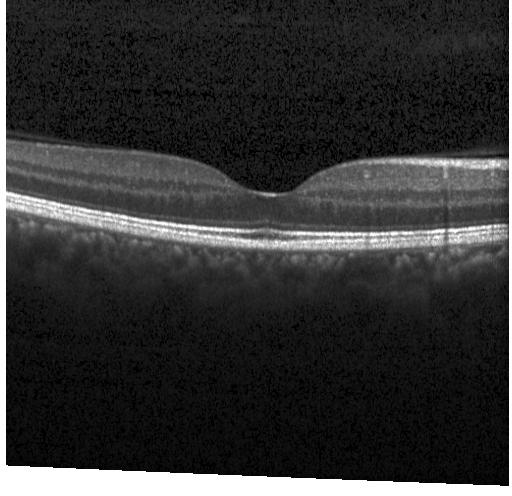

Fovea-centered · OCT line scan · SD-OCT
No CNV, DME, or drusen.